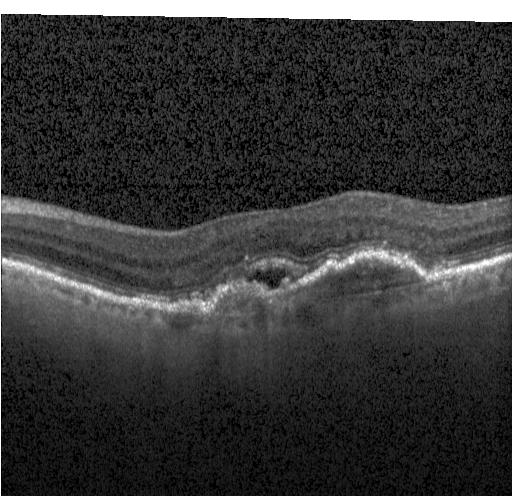 Diagnosis: CNV.